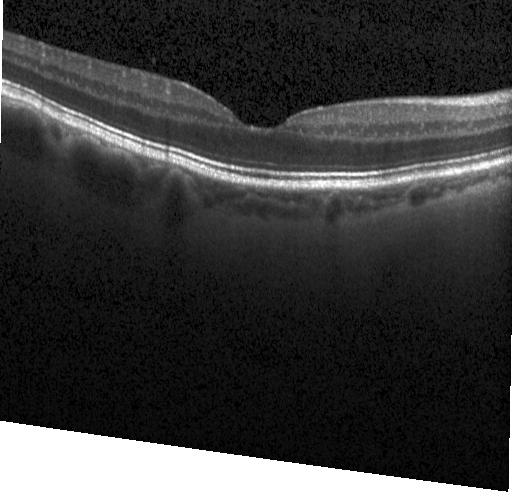 OCT B-scan; acquired on a Heidelberg Spectralis; spectral-domain OCT
The scan shows no choroidal neovascularization, diabetic macular edema, or drusen.